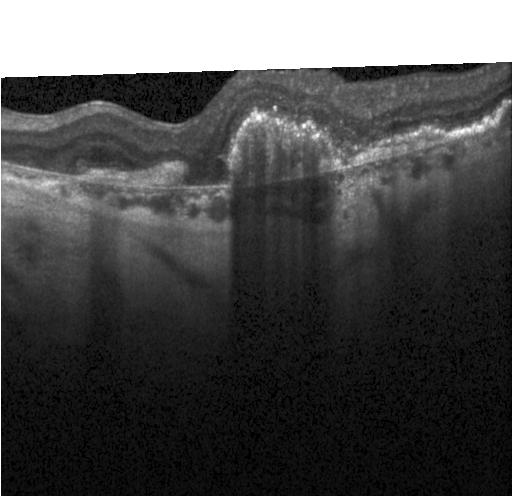
Retinal OCT cross-section · spectral-domain OCT · Heidelberg Spectralis OCT system · fovea-centered. Assessment: CNV.